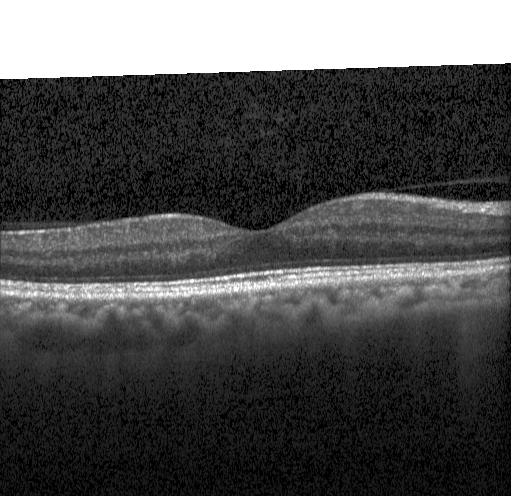 Heidelberg Spectralis OCT system. Optical coherence tomography scan. Through the macula.
Diagnosis: neither choroidal neovascularization, diabetic macular edema, nor drusen.